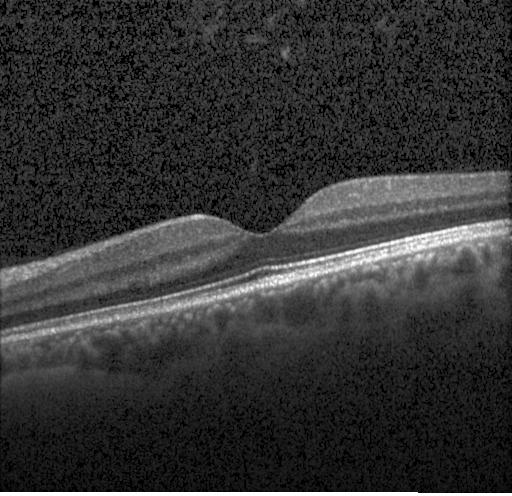

Spectral-domain OCT; Heidelberg Spectralis; fovea-centered; optical coherence tomography scan.
Diagnosis: no evidence of choroidal neovascularization, diabetic macular edema, or drusen.